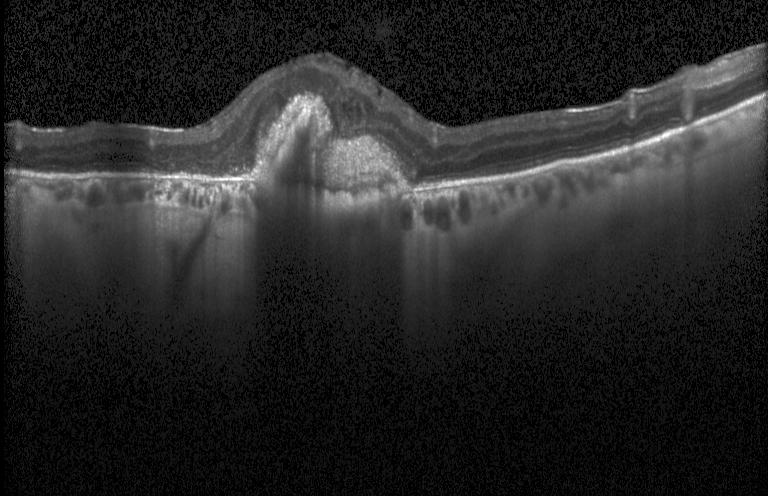
OCT B-scan showing CNV.